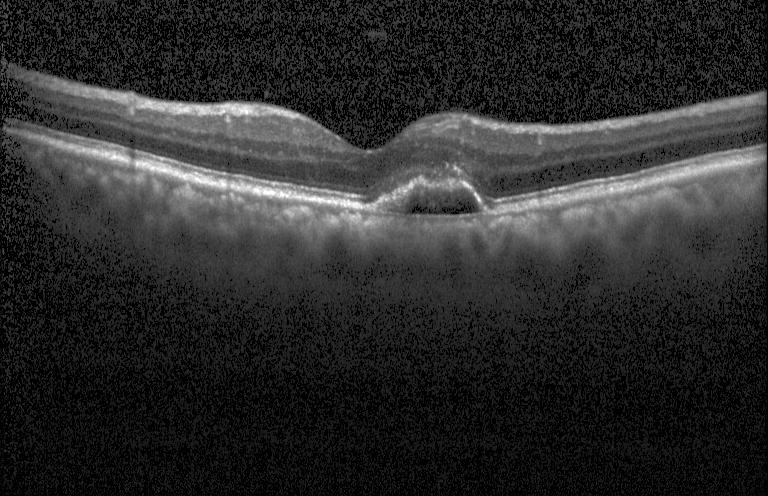 A choroidal neovascular membrane.